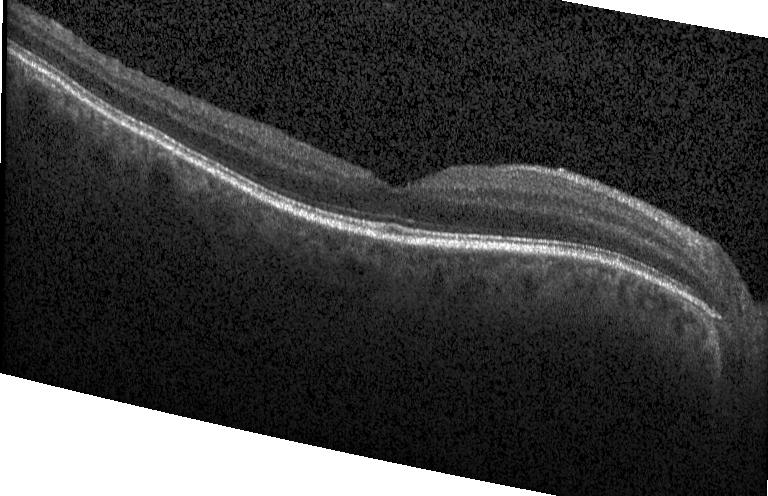
Instrument: Heidelberg Spectralis. Spectral-domain optical coherence tomography. Retinal OCT B-scan. Through the macula
Macular OCT: no CNV, no DME, and no drusen.